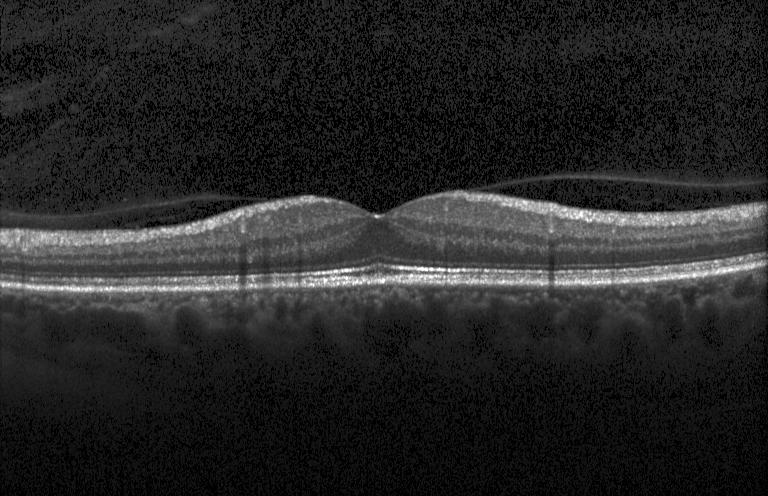

Retinal OCT cross-section — Macular OCT: no choroidal neovascularization, diabetic macular edema, or drusen.